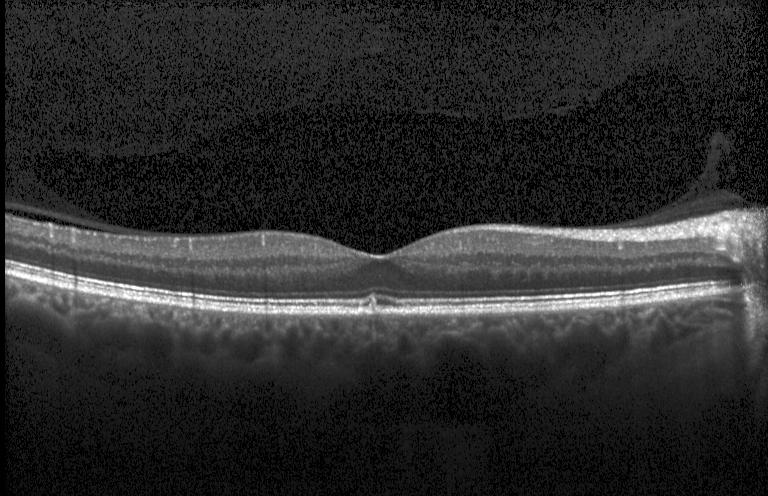

Macular OCT demonstrating drusen.